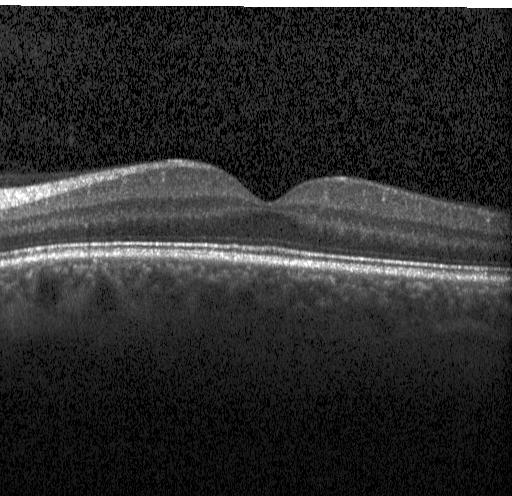

Retinal OCT B-scan, fovea-centered, Heidelberg Spectralis, SD-OCT — Macular OCT: no CNV, no DME, and no drusen.